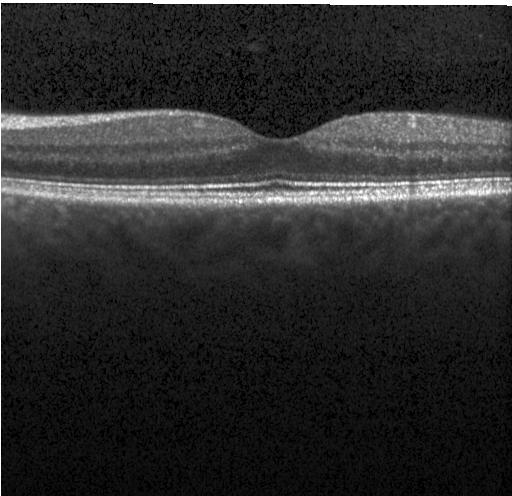

Centered on the fovea; Heidelberg Spectralis; OCT B-scan.
Dx: neither choroidal neovascularization, diabetic macular edema, nor drusen.